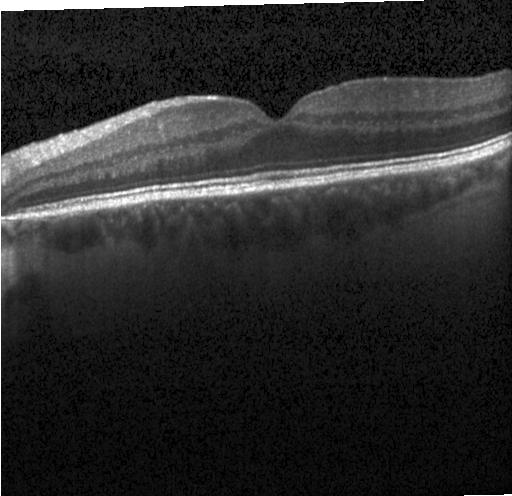 Acquired on a Heidelberg Spectralis; optical coherence tomography B-scan; spectral-domain optical coherence tomography — Assessment: no evidence of CNV, DME, or drusen.